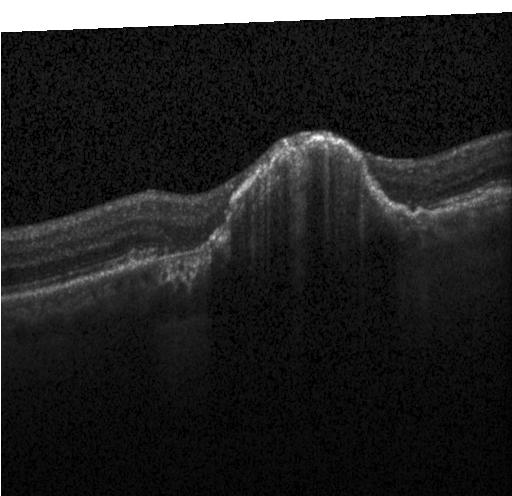 Macular OCT: choroidal neovascularization (CNV).